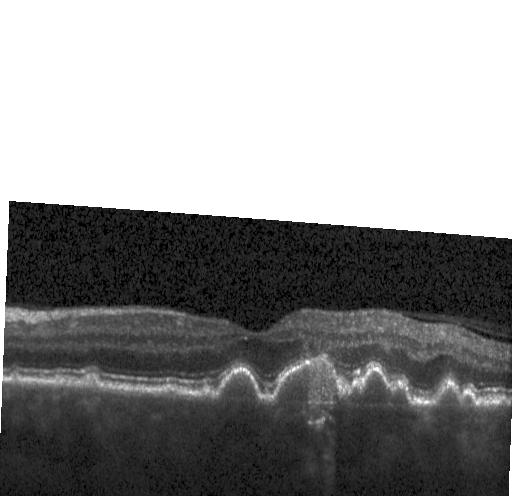 Finding: sub-RPE drusenoid deposits.